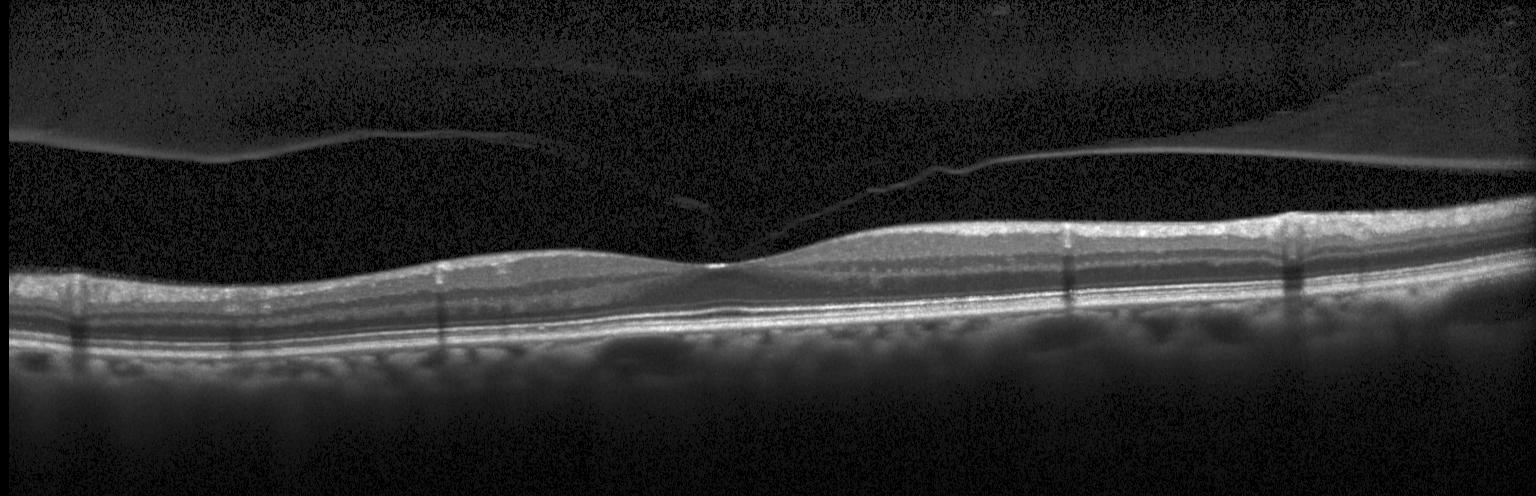

Fovea-centered · retinal OCT cross-section · spectral-domain optical coherence tomography
OCT finding: neither choroidal neovascularization, diabetic macular edema, nor drusen.